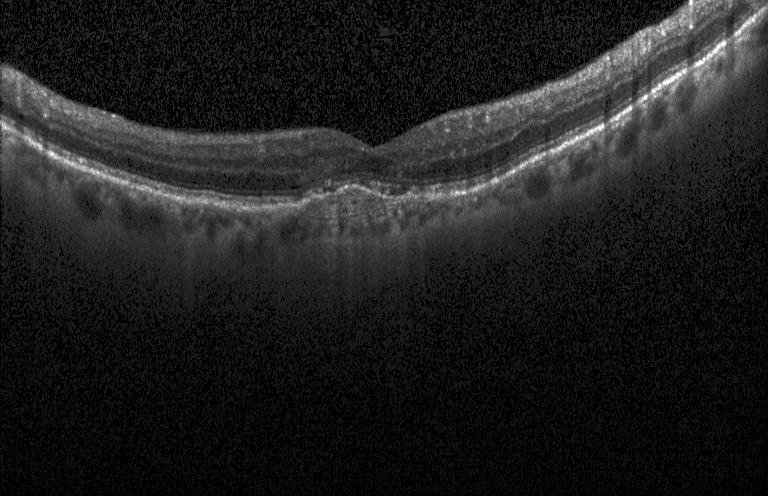
Optical coherence tomography scan — Finding: choroidal neovascularization (CNV).